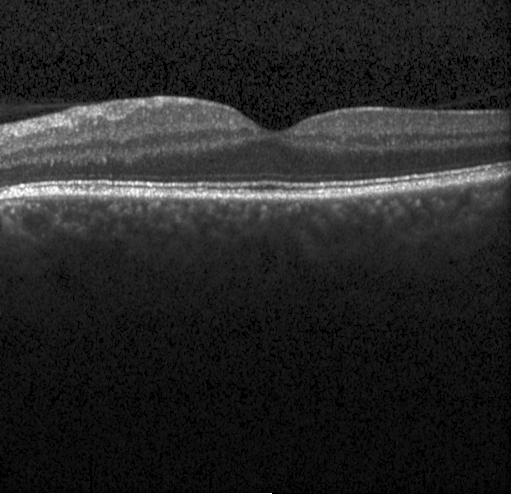 Spectral-domain OCT · optical coherence tomography B-scan — Diagnosis: no choroidal neovascularization, diabetic macular edema, or drusen.